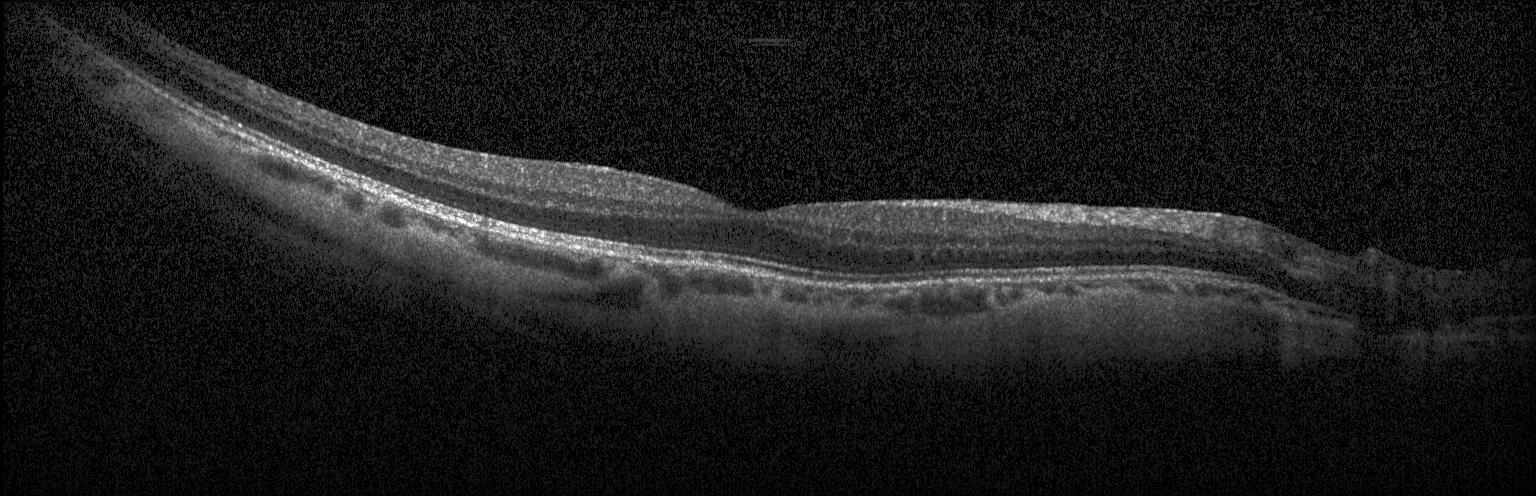
Macular scan · optical coherence tomography B-scan
Diagnosis: no CNV, no DME, and no drusen.